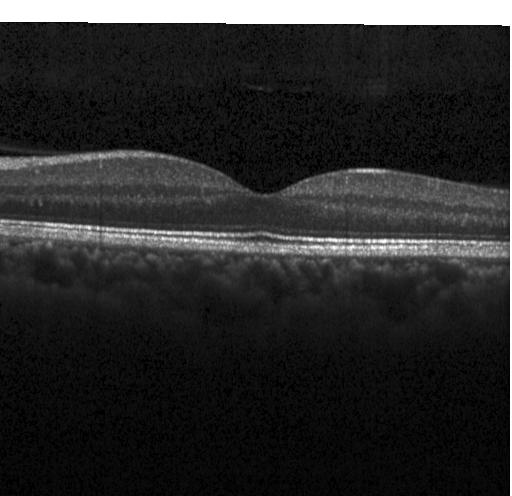

Optical coherence tomography B-scan
Macular OCT: no evidence of CNV, DME, or drusen.